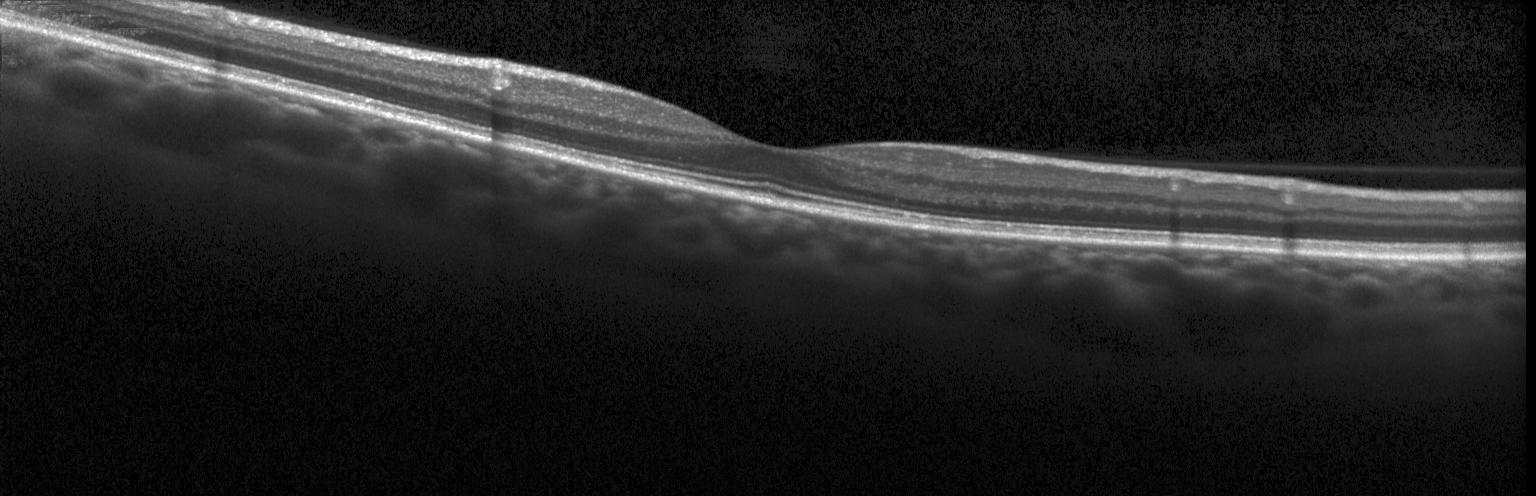
Retinal OCT B-scan — Impression: no CNV, no DME, and no drusen.